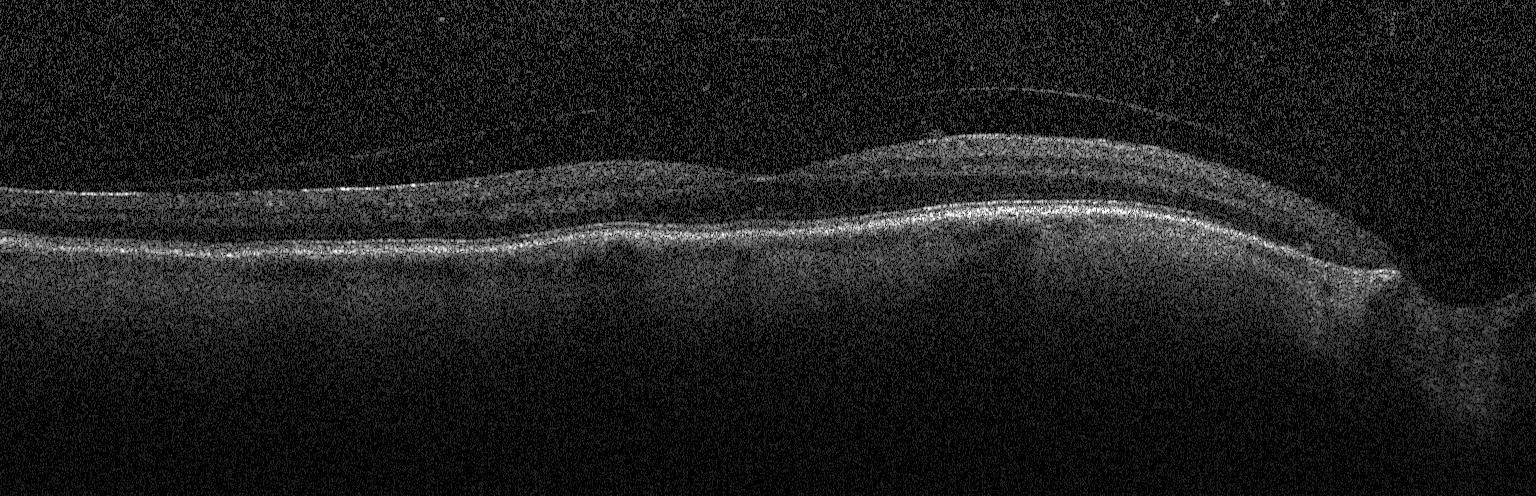 Optical coherence tomography B-scan.
Assessment: neither choroidal neovascularization, diabetic macular edema, nor drusen.